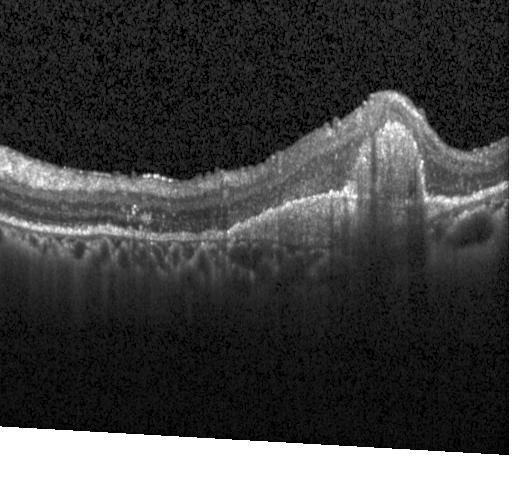

Optical coherence tomography B-scan — This B-scan demonstrates a choroidal neovascular membrane.